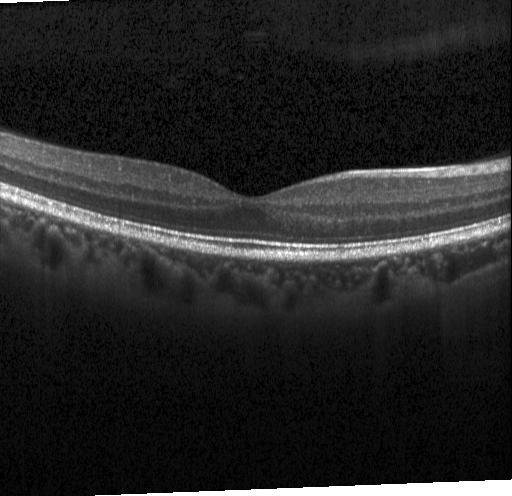
OCT line scan, spectral-domain optical coherence tomography, fovea-centered — No choroidal neovascularization, diabetic macular edema, or drusen.